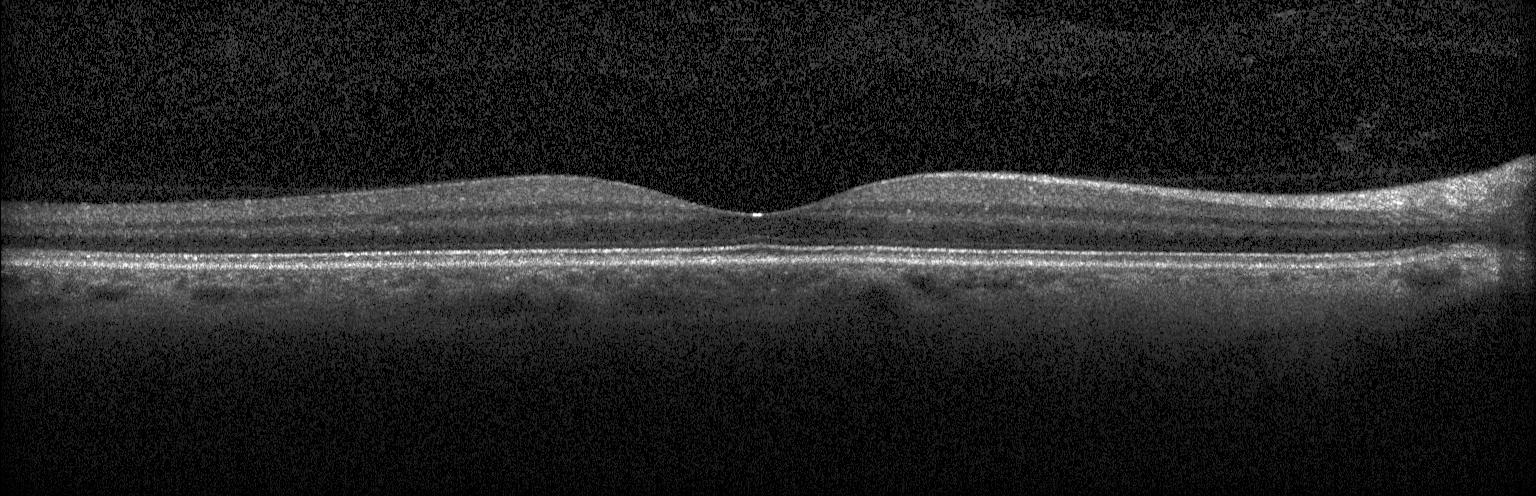
Impression: no evidence of choroidal neovascularization, diabetic macular edema, or drusen.